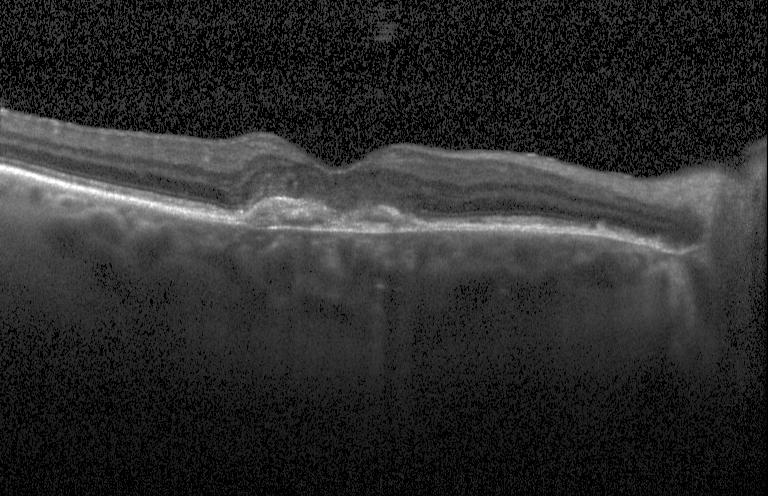
Spectral-domain optical coherence tomography, retinal OCT B-scan. This B-scan demonstrates a choroidal neovascular membrane.